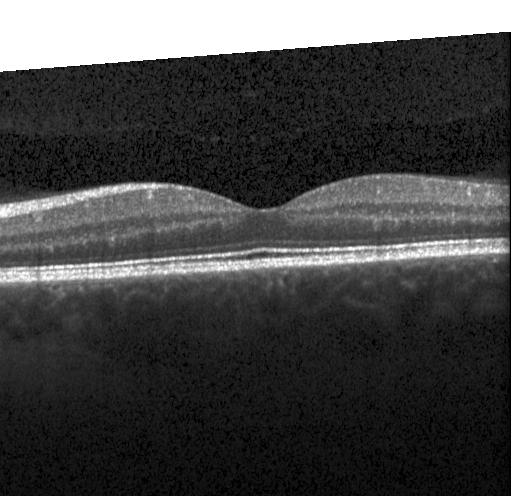

SD-OCT, retinal OCT B-scan, Heidelberg Spectralis.
Dx: no evidence of choroidal neovascularization, diabetic macular edema, or drusen.